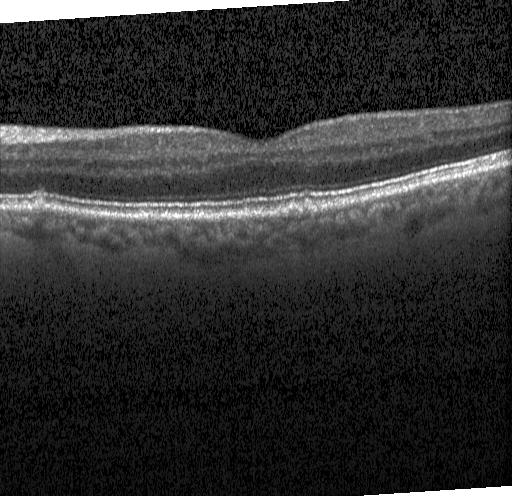 OCT line scan
Impression: drusen.